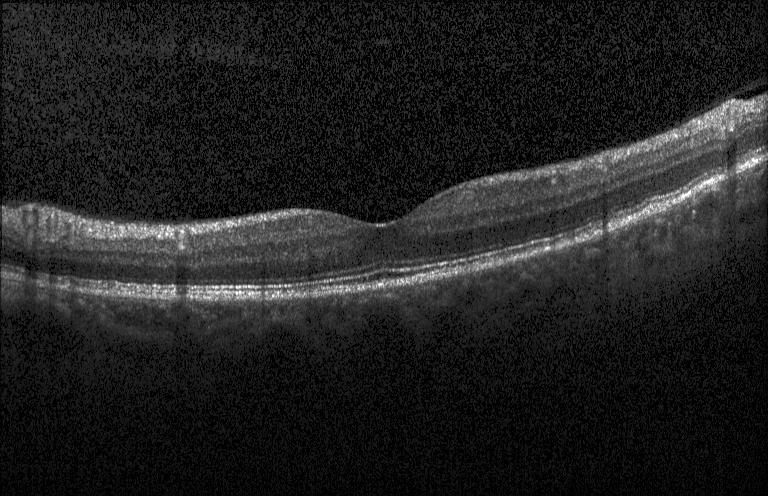 Optical coherence tomography scan; fovea-centered; SD-OCT
Assessment: drusen.